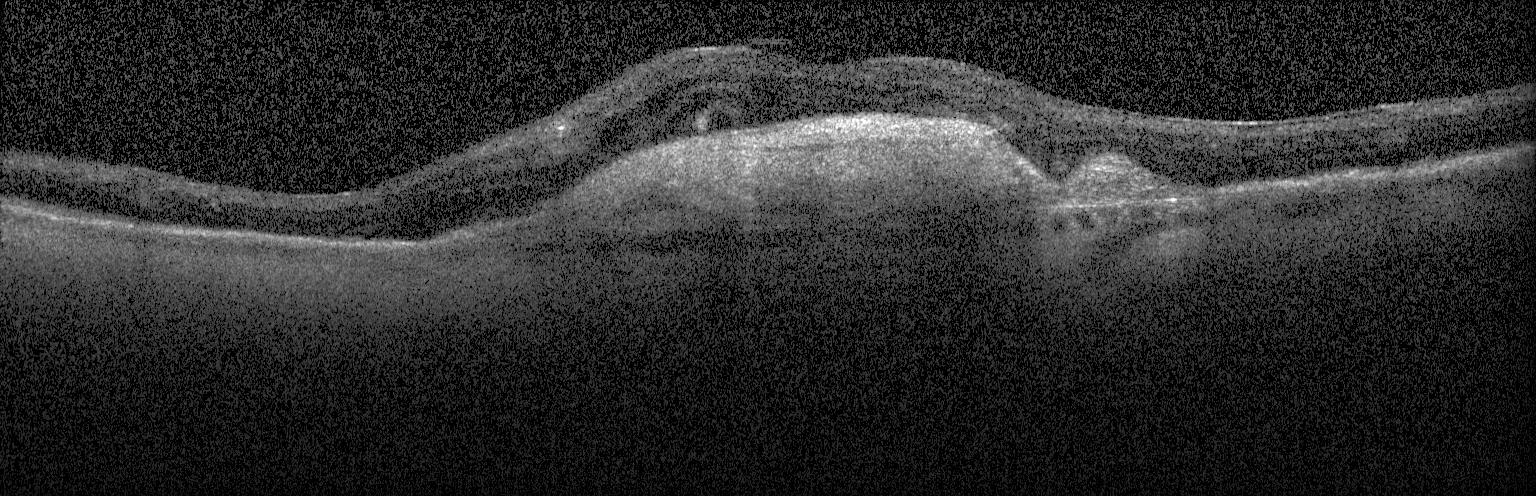

OCT line scan.
Finding: a choroidal neovascular membrane.